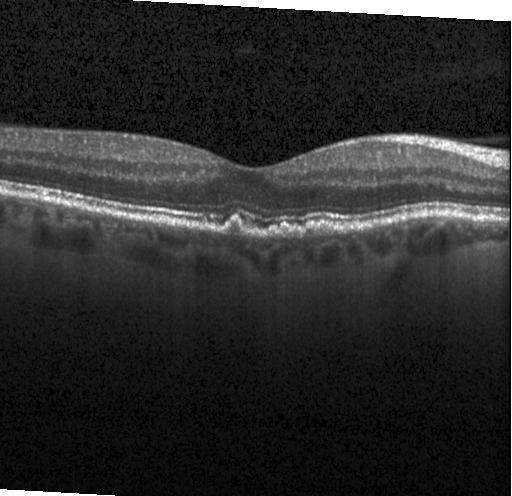 OCT finding: drusen.